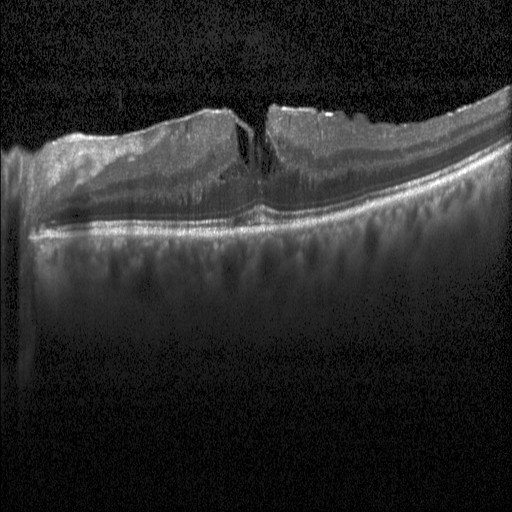

OCT line scan · Heidelberg Spectralis OCT system · horizontal scan through the fovea · spectral-domain optical coherence tomography — This B-scan demonstrates diabetic macular edema (DME).